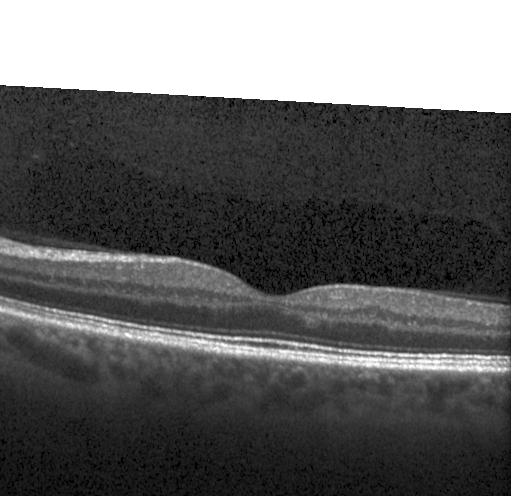 Horizontal scan through the fovea. Spectral-domain optical coherence tomography. OCT B-scan.
The scan shows no choroidal neovascularization, no diabetic macular edema, and no drusen.